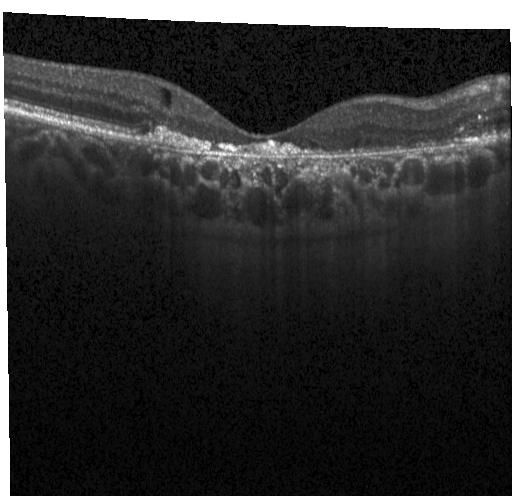
OCT scan showing choroidal neovascularization.